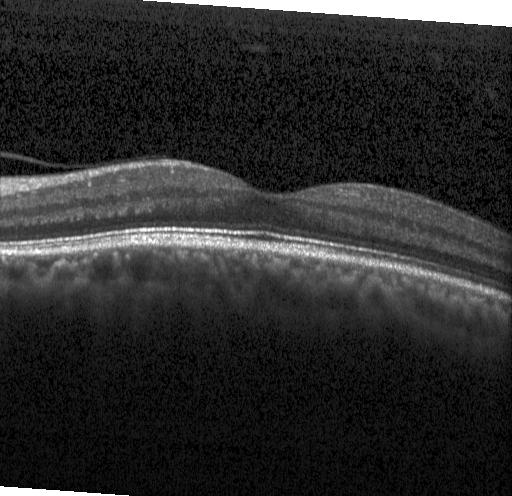
Retinal OCT B-scan, Heidelberg Spectralis OCT system.
The scan shows no choroidal neovascularization, diabetic macular edema, or drusen.